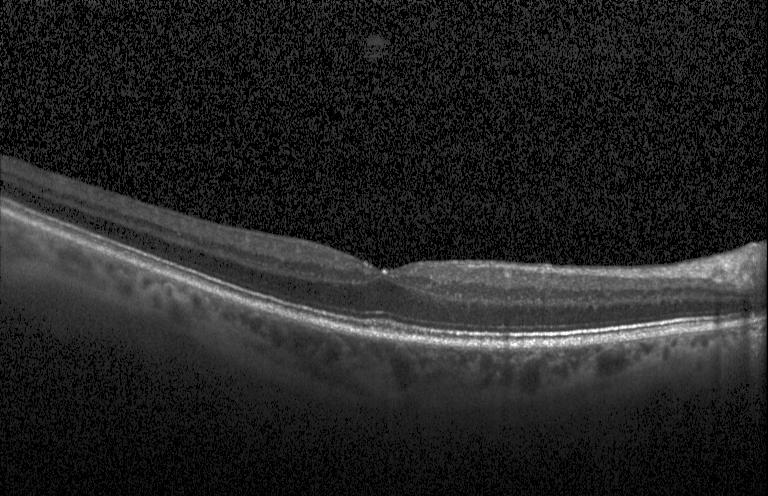
Spectral-domain optical coherence tomography, Heidelberg Spectralis OCT system, optical coherence tomography scan, through the macula — Finding: no evidence of CNV, DME, or drusen.